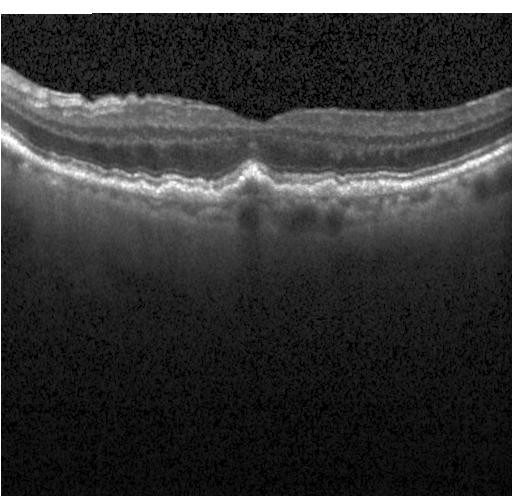
Assessment: a choroidal neovascular membrane.